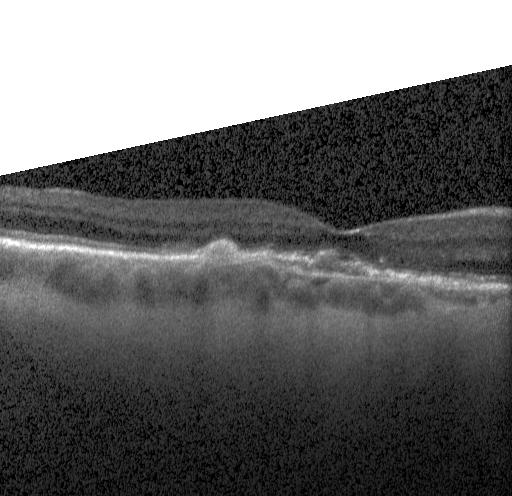 Instrument: Heidelberg Spectralis. Horizontal scan through the fovea. Optical coherence tomography scan. SD-OCT — Macular OCT: a choroidal neovascular membrane.